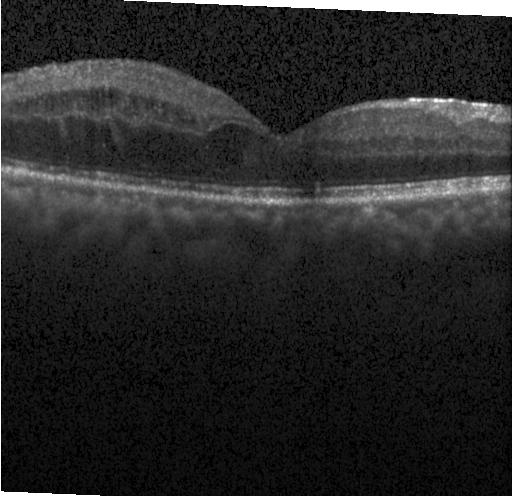 Dx: DME.